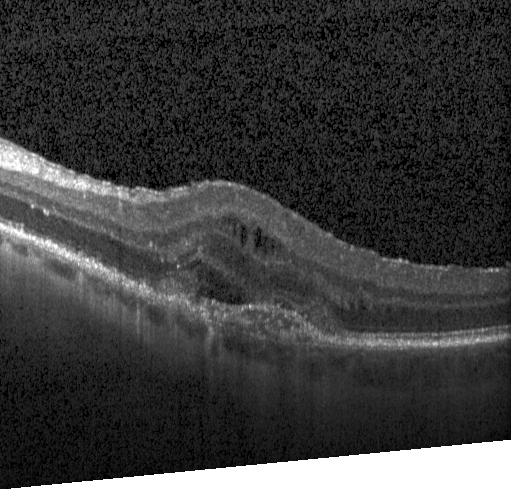

Acquired on a Heidelberg Spectralis. SD-OCT. Retinal OCT B-scan.
Impression: CNV.